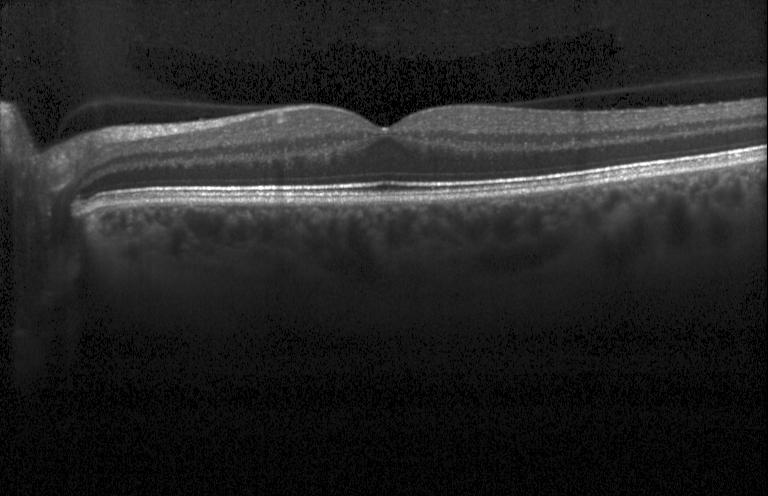 OCT finding: no choroidal neovascularization, diabetic macular edema, or drusen.